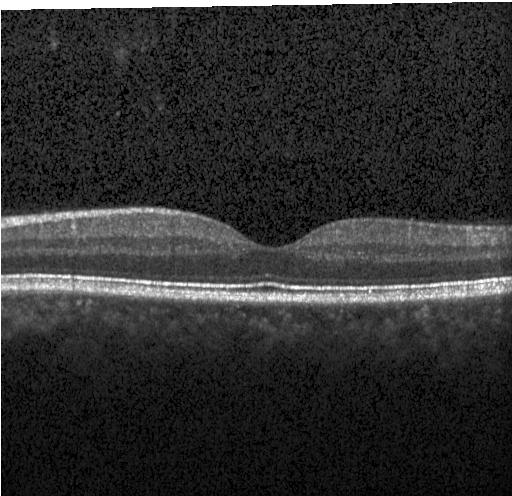

Macular scan · retinal OCT B-scan · spectral-domain optical coherence tomography · instrument: Heidelberg Spectralis. Diagnosis: neither CNV, DME, nor drusen.